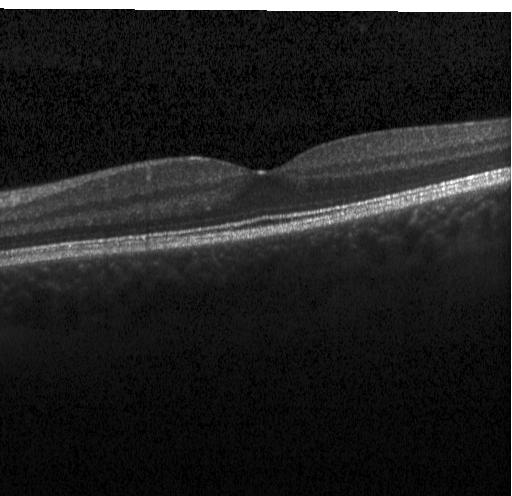

Retinal OCT cross-section showing no CNV, DME, or drusen.